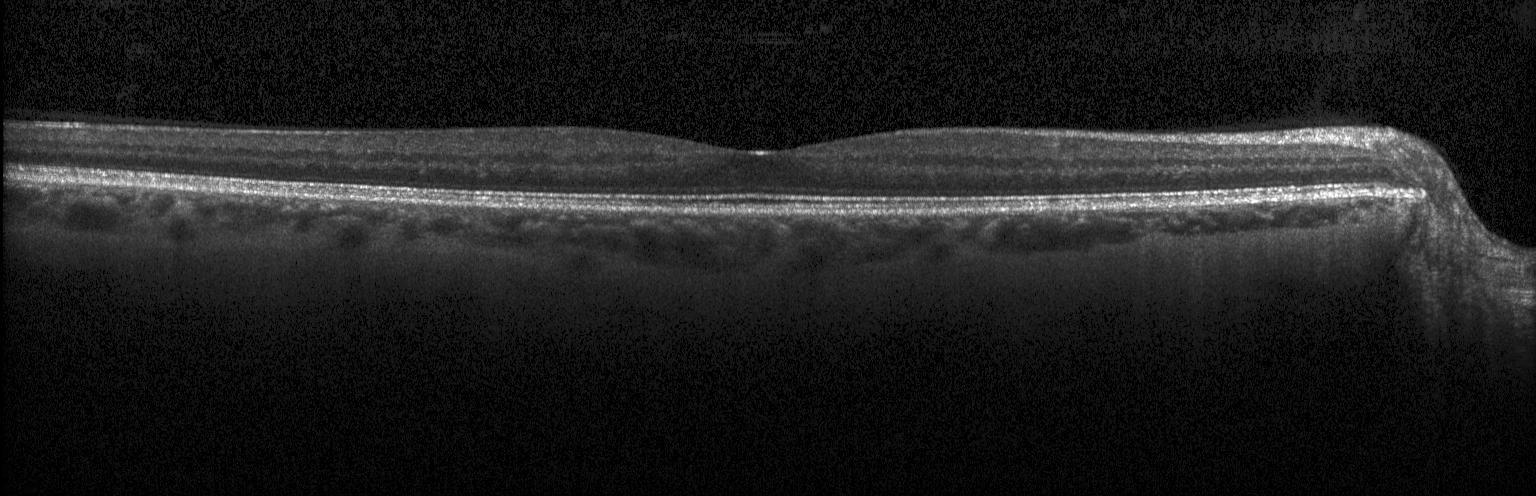
Dx: no choroidal neovascularization, diabetic macular edema, or drusen.